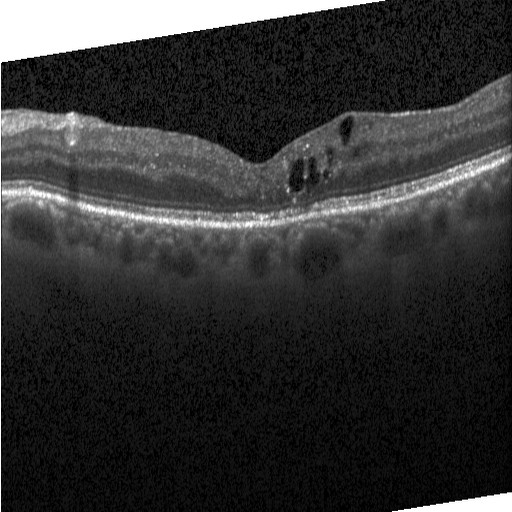
Through the macula. Heidelberg Spectralis. Optical coherence tomography B-scan
Dx: DME.